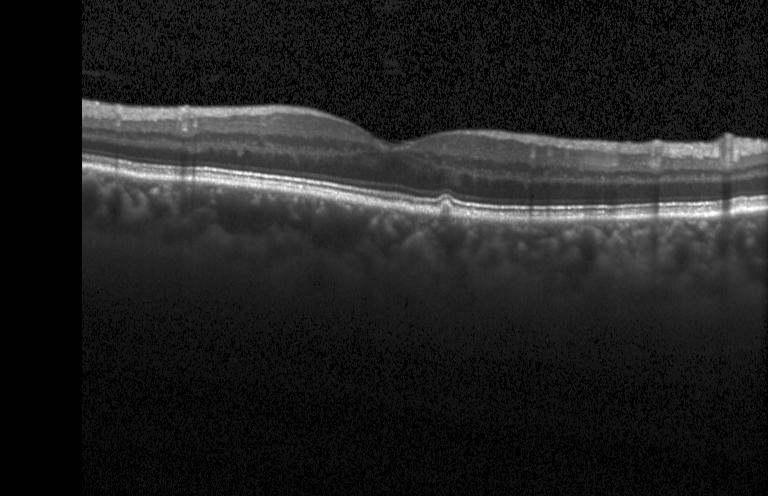
Spectral-domain optical coherence tomography; horizontal scan through the fovea; retinal OCT cross-section
Assessment: multiple drusen.